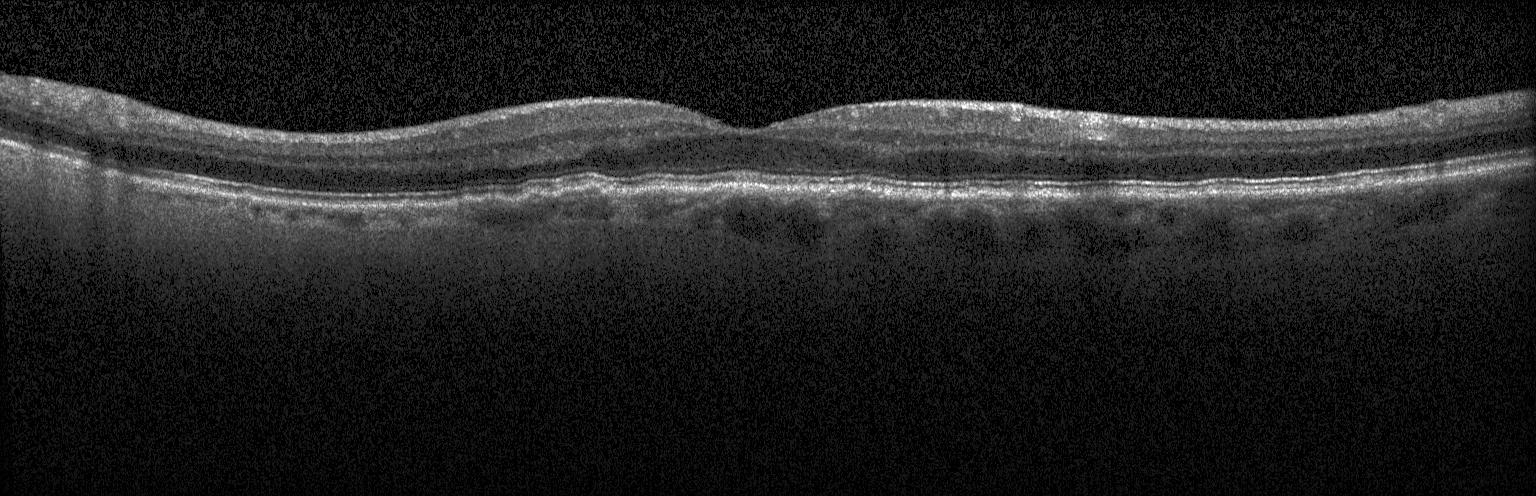
Spectral-domain OCT, optical coherence tomography scan, Heidelberg Spectralis, fovea-centered. The scan shows drusen.